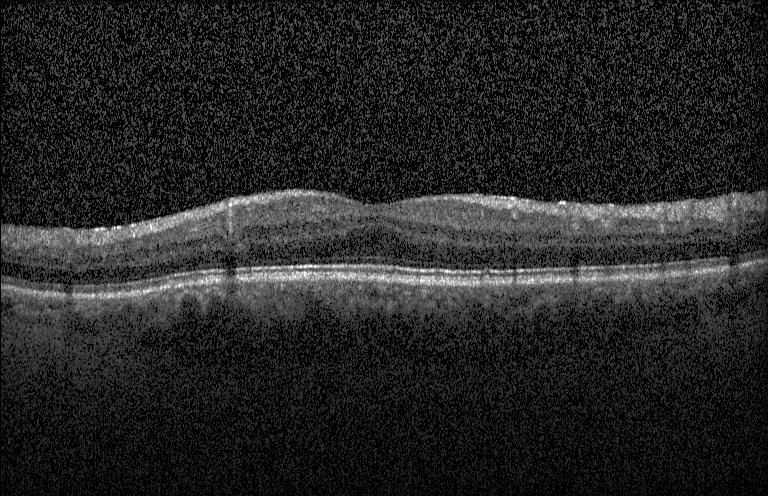 Retinal OCT B-scan — Macular OCT: neither choroidal neovascularization, diabetic macular edema, nor drusen.